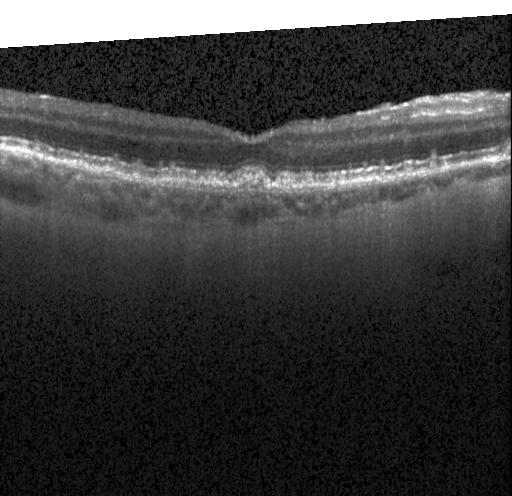 Impression: drusen.